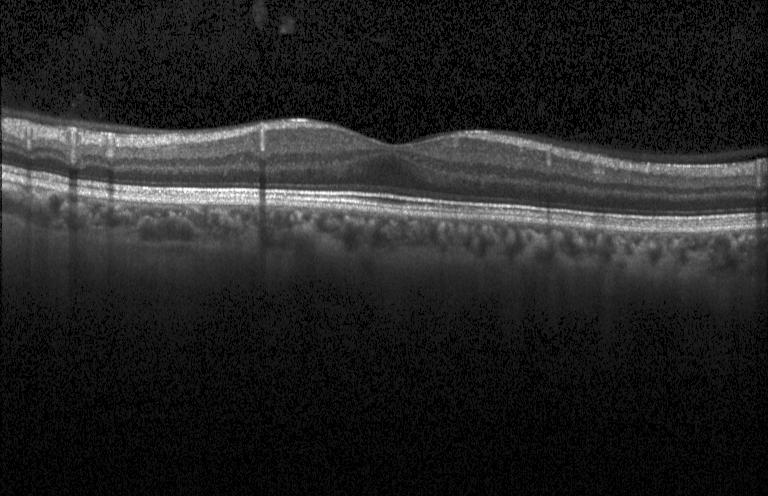 No choroidal neovascularization, diabetic macular edema, or drusen.